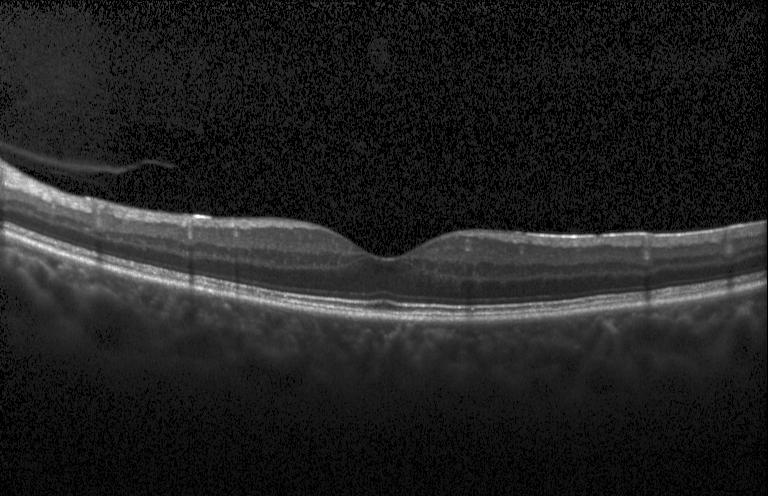 Horizontal scan through the fovea. Optical coherence tomography scan.
Macular OCT: neither CNV, DME, nor drusen.